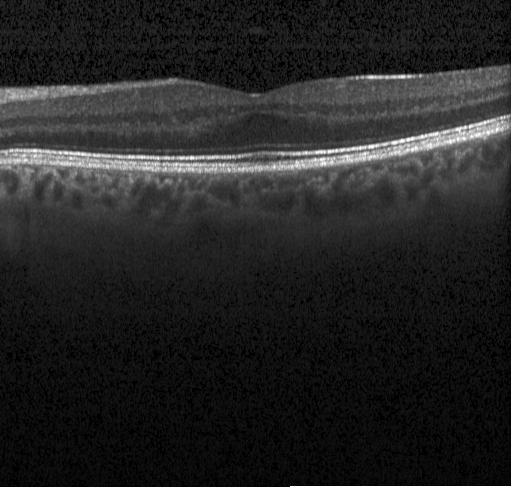 Retinal OCT cross-section.
The scan shows neither choroidal neovascularization, diabetic macular edema, nor drusen.